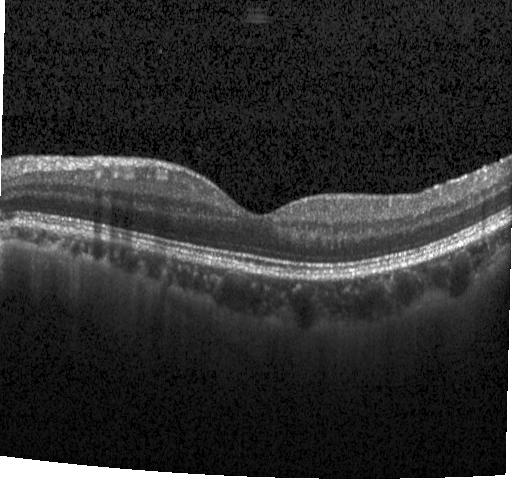

OCT line scan, macular scan, SD-OCT, Heidelberg Spectralis.
Finding: neither choroidal neovascularization, diabetic macular edema, nor drusen.